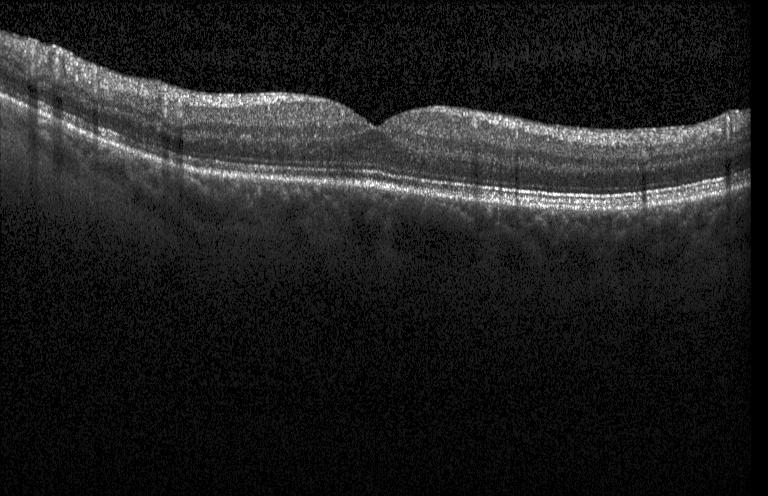
OCT B-scan; Heidelberg Spectralis.
Diagnosis: no CNV, no DME, and no drusen.